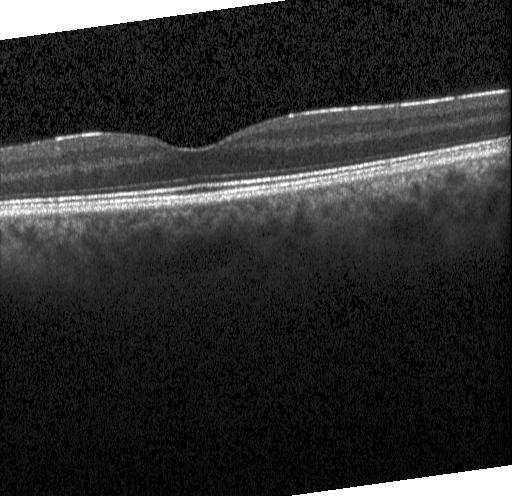

Retinal OCT B-scan. Fovea-centered
Neither choroidal neovascularization, diabetic macular edema, nor drusen.